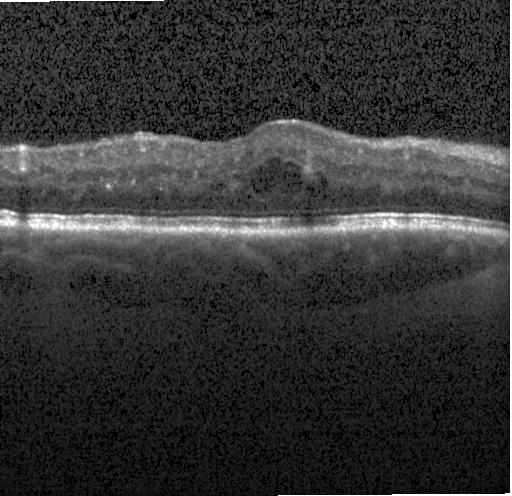

Finding: DME.